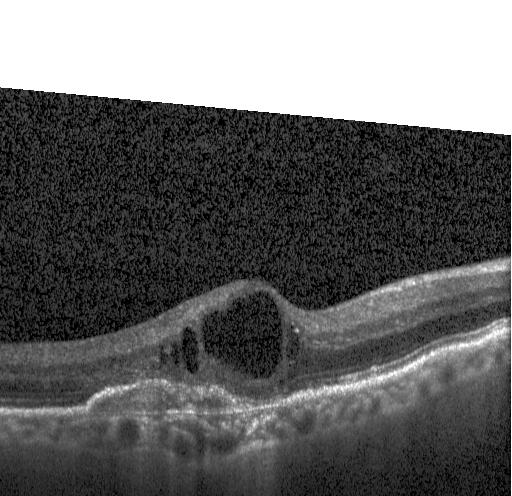
Centered on the fovea, optical coherence tomography scan, SD-OCT, acquired on a Heidelberg Spectralis.
Finding: CNV.